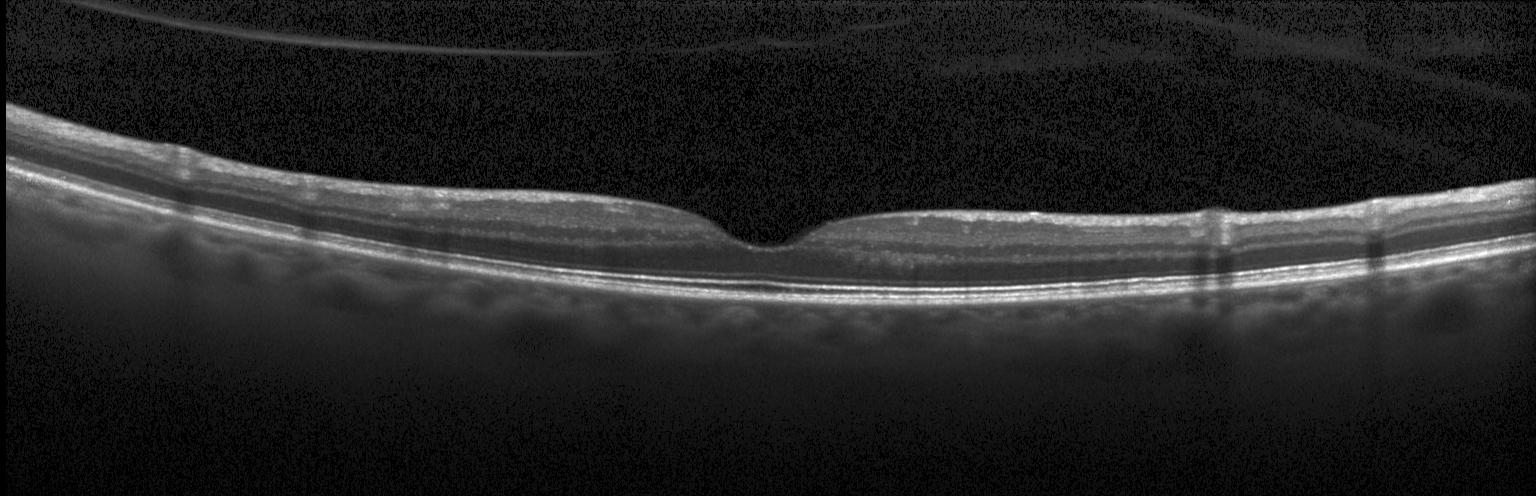

Retinal OCT cross-section; acquired on a Heidelberg Spectralis.
The scan shows no evidence of CNV, DME, or drusen.